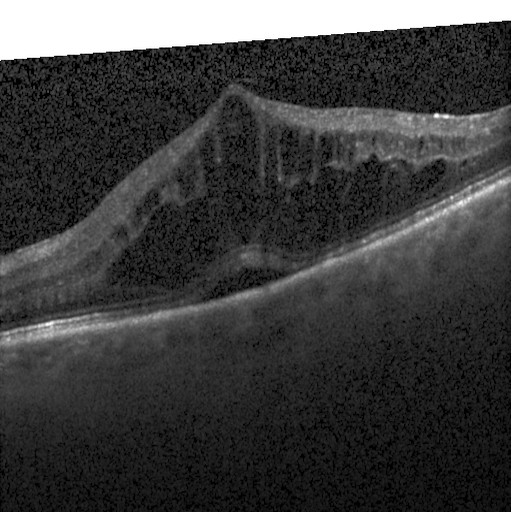
OCT line scan.
Assessment: diabetic macular edema (DME).